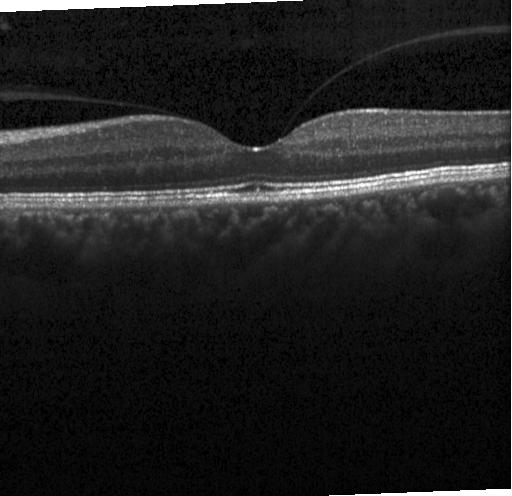 Horizontal scan through the fovea · Heidelberg Spectralis · spectral-domain OCT · optical coherence tomography B-scan. Assessment: no CNV, DME, or drusen.